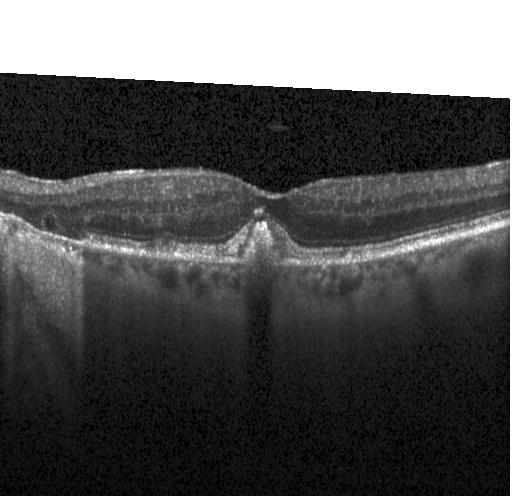 Acquired on a Heidelberg Spectralis; optical coherence tomography B-scan
A choroidal neovascular membrane.